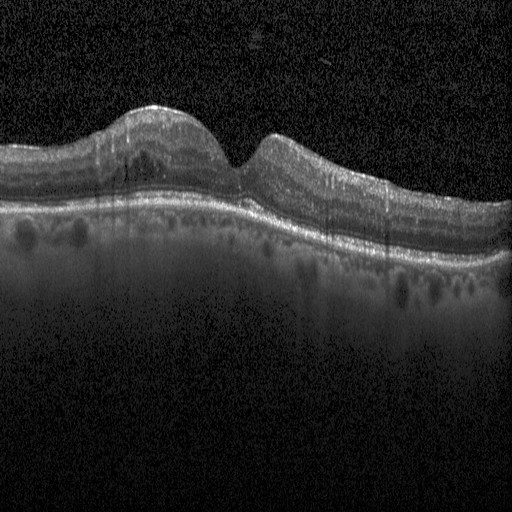 OCT B-scan showing diabetic macular edema.